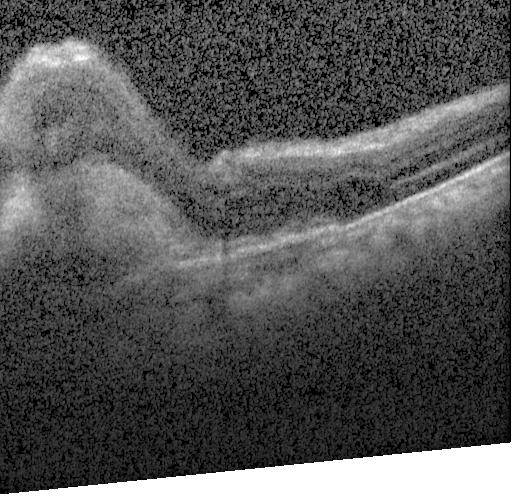
Spectral-domain OCT · retinal OCT cross-section — A choroidal neovascular membrane.